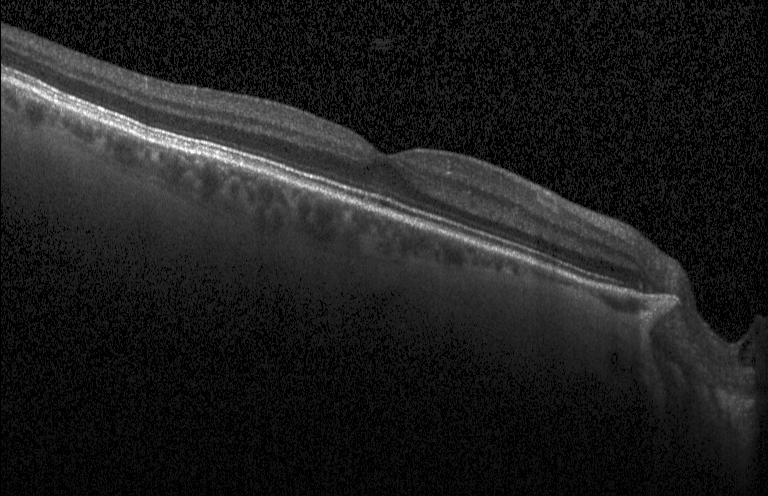
Impression: neither choroidal neovascularization, diabetic macular edema, nor drusen.